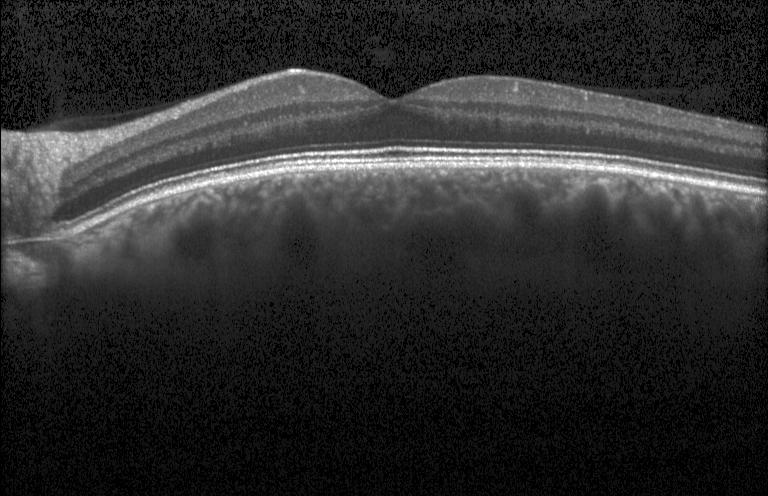

Impression: no choroidal neovascularization, no diabetic macular edema, and no drusen.